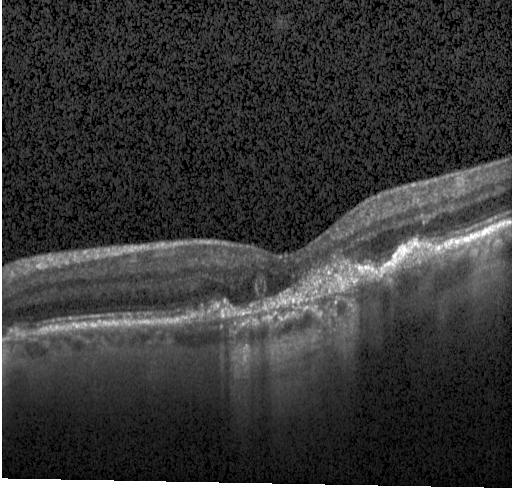
Through the macula. Spectral-domain optical coherence tomography. Acquired on a Heidelberg Spectralis. OCT line scan
Impression: a choroidal neovascular membrane.